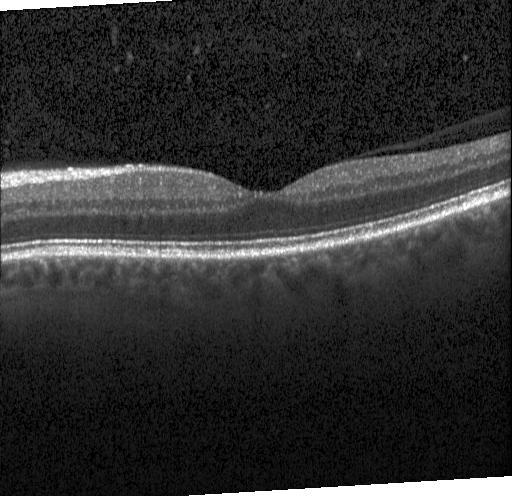
The scan shows no CNV, DME, or drusen.